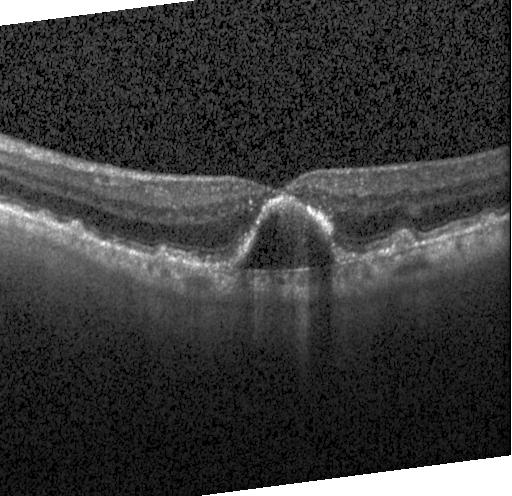
Instrument: Heidelberg Spectralis. Optical coherence tomography B-scan. Through the macula — Impression: choroidal neovascularization.